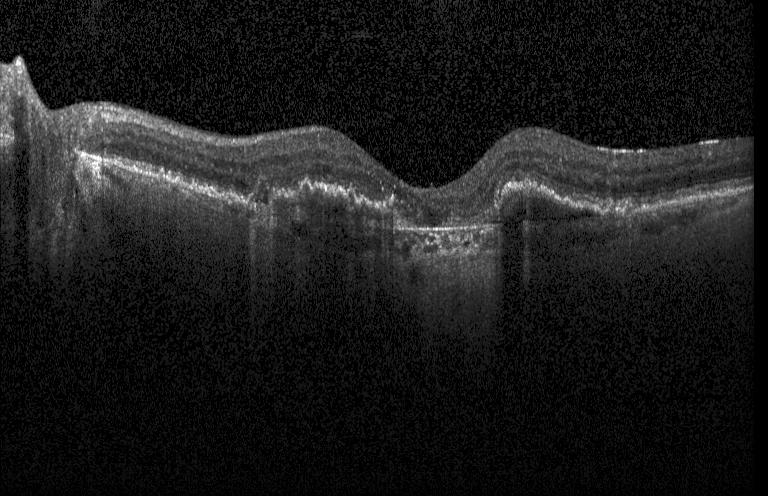
Centered on the fovea, OCT B-scan.
Finding: a choroidal neovascular membrane.